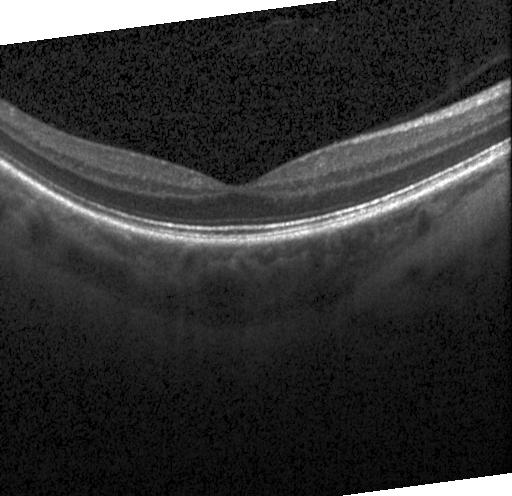

Instrument: Heidelberg Spectralis; spectral-domain optical coherence tomography; optical coherence tomography scan
Diagnosis: no evidence of choroidal neovascularization, diabetic macular edema, or drusen.